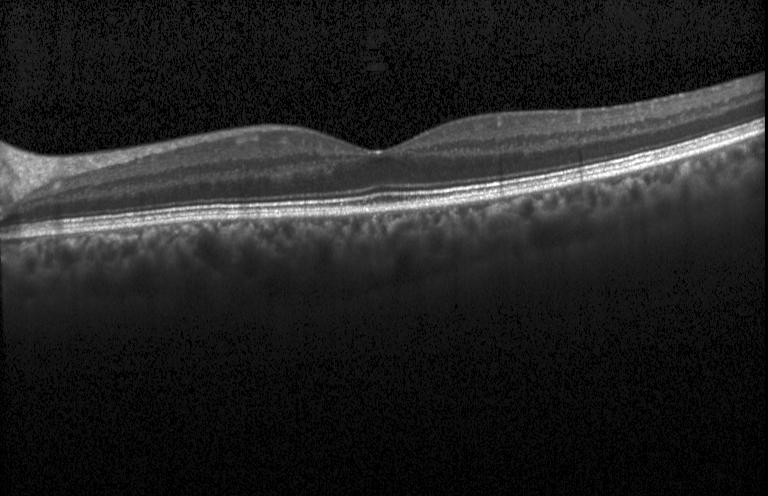

Retinal OCT B-scan; spectral-domain optical coherence tomography; fovea-centered
Diagnosis: neither choroidal neovascularization, diabetic macular edema, nor drusen.